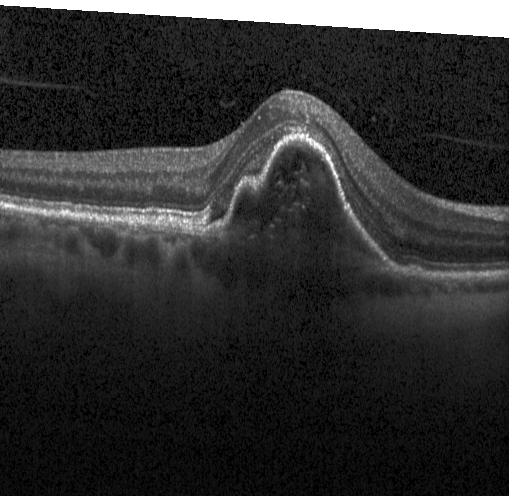
OCT finding: choroidal neovascularization (CNV).